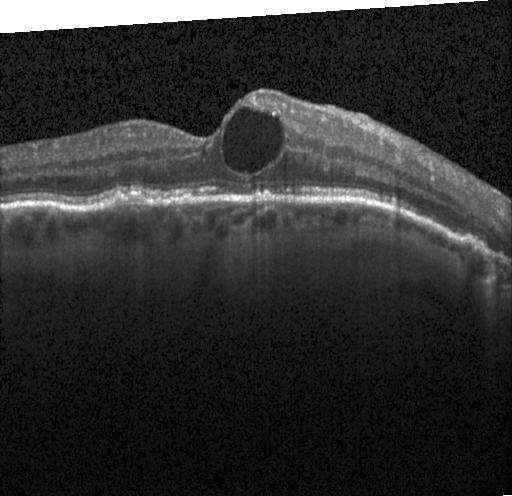

Impression: CNV.